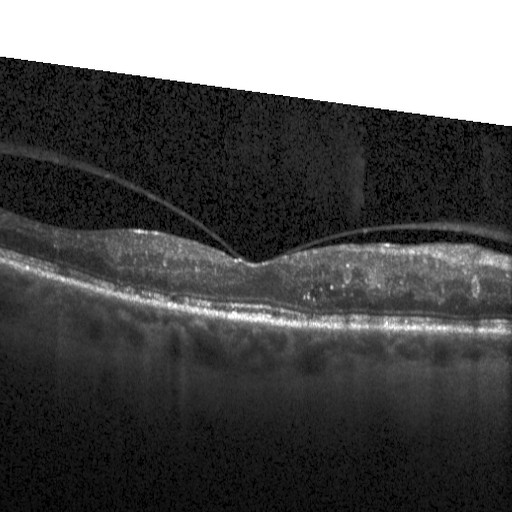 SD-OCT · optical coherence tomography scan · centered on the fovea
Dx: diabetic macular edema.